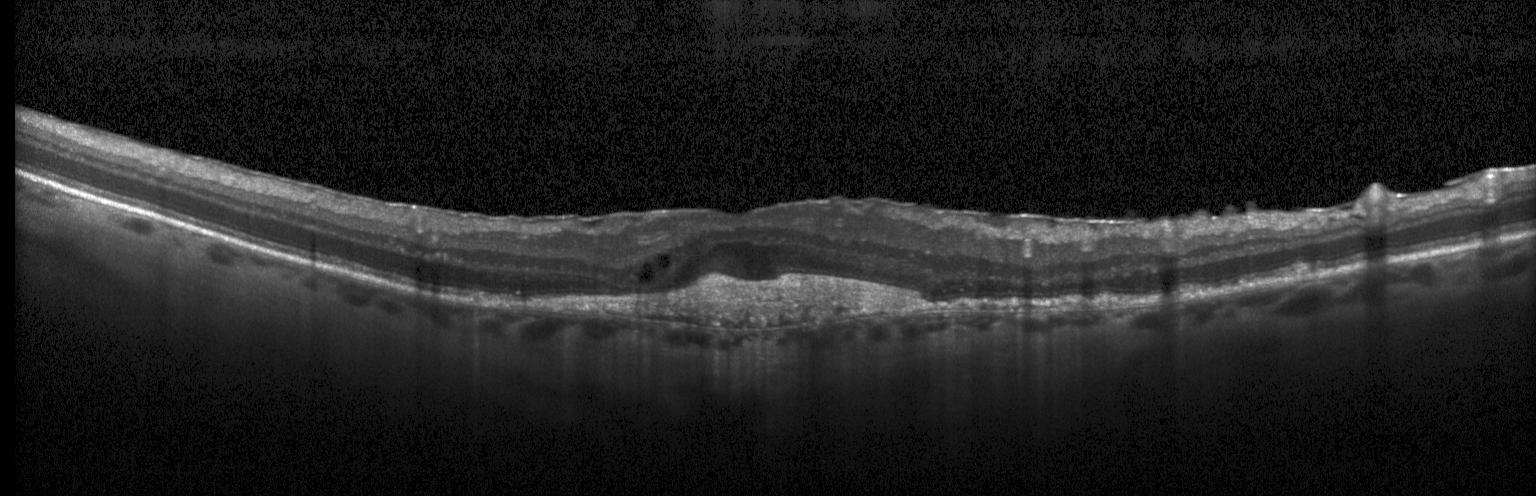

Macular OCT: choroidal neovascularization (CNV).